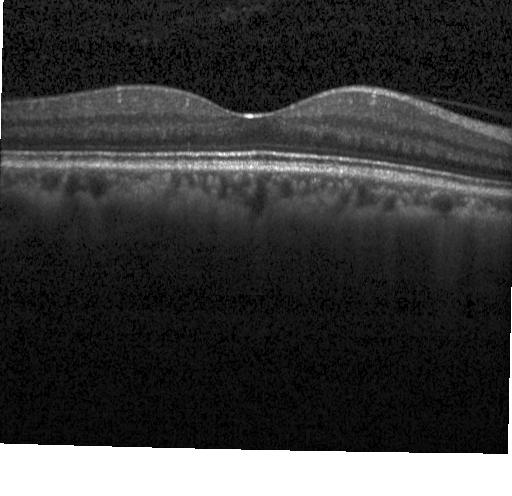
Horizontal scan through the fovea · spectral-domain optical coherence tomography · instrument: Heidelberg Spectralis · OCT line scan. Impression: no choroidal neovascularization, no diabetic macular edema, and no drusen.